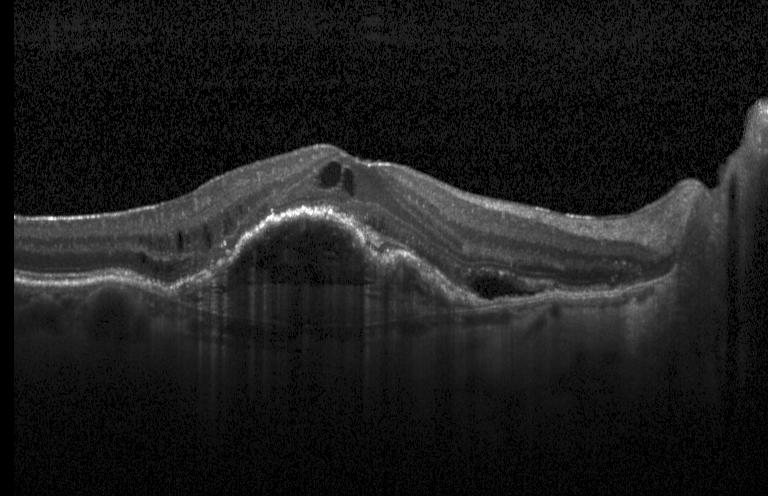

OCT B-scan · horizontal scan through the fovea · Heidelberg Spectralis.
Assessment: a choroidal neovascular membrane.